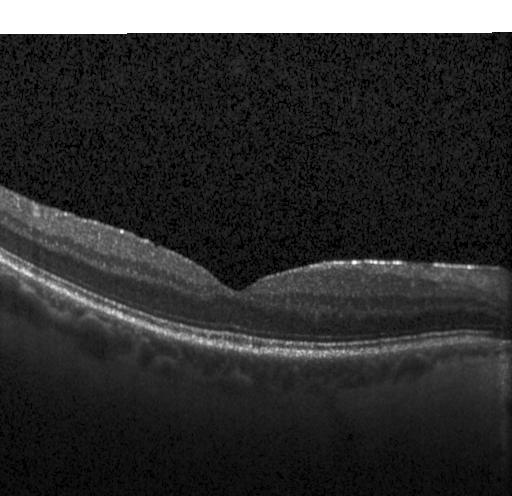 OCT finding: no evidence of choroidal neovascularization, diabetic macular edema, or drusen.